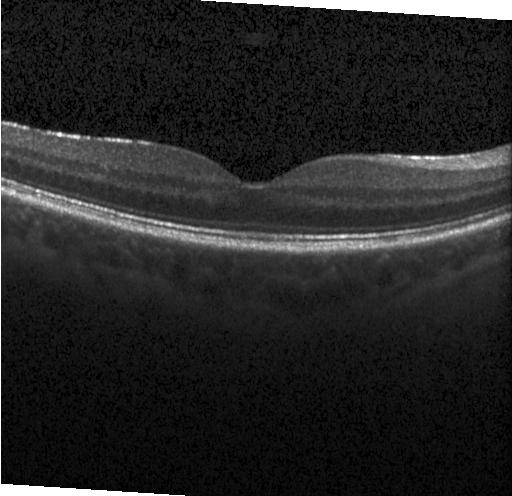 OCT B-scan showing no choroidal neovascularization, no diabetic macular edema, and no drusen.